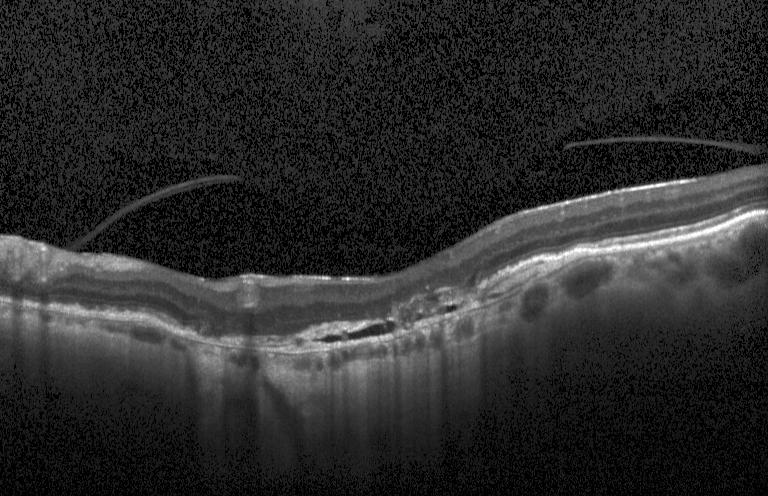
Optical coherence tomography scan, horizontal scan through the fovea, SD-OCT, Heidelberg Spectralis OCT system — Finding: choroidal neovascularization (CNV).